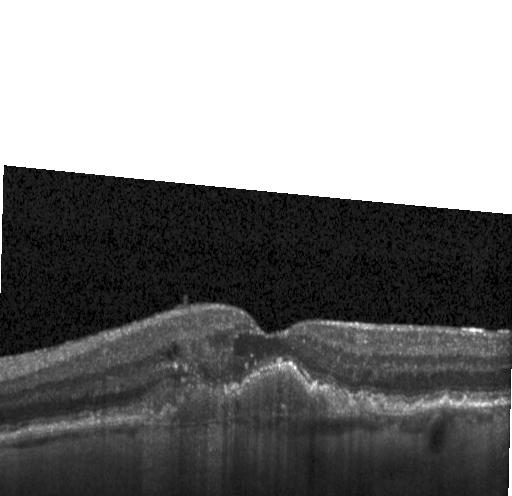 Spectral-domain optical coherence tomography; macular scan; retinal OCT B-scan; Heidelberg Spectralis OCT system — Diagnosis: choroidal neovascularization.